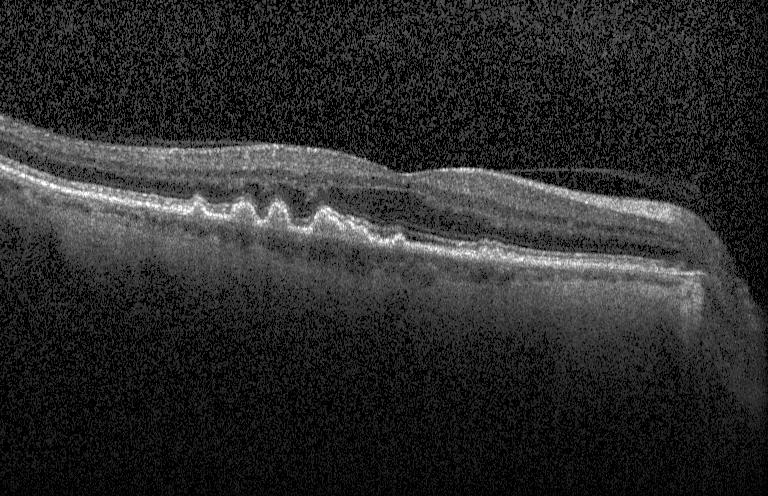 OCT B-scan — Drusen.